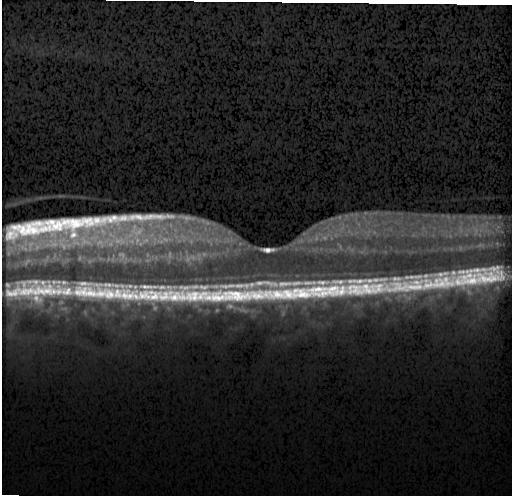
Optical coherence tomography B-scan — Diagnosis: no evidence of choroidal neovascularization, diabetic macular edema, or drusen.